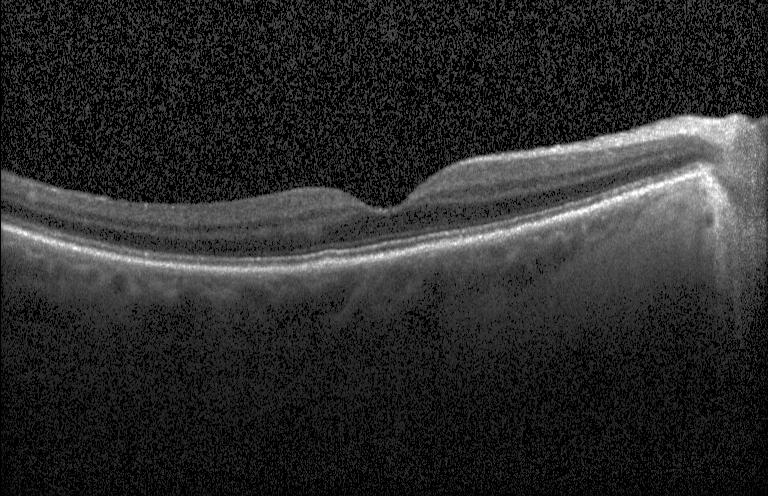 Finding: no CNV, no DME, and no drusen.